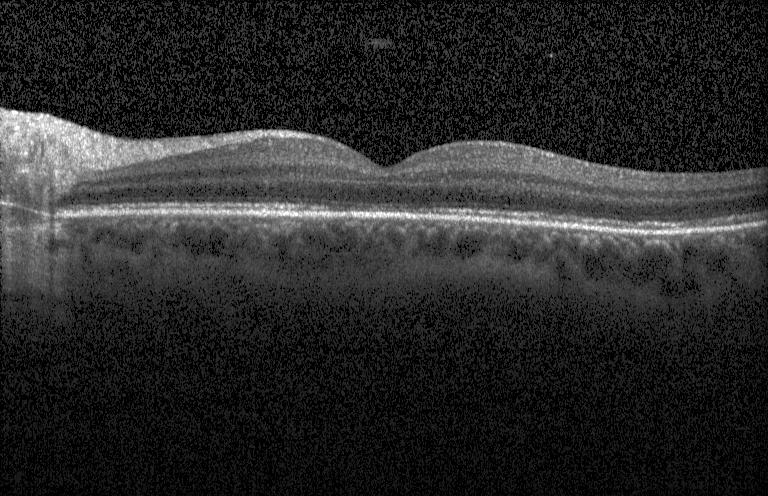

OCT line scan. Neither choroidal neovascularization, diabetic macular edema, nor drusen.